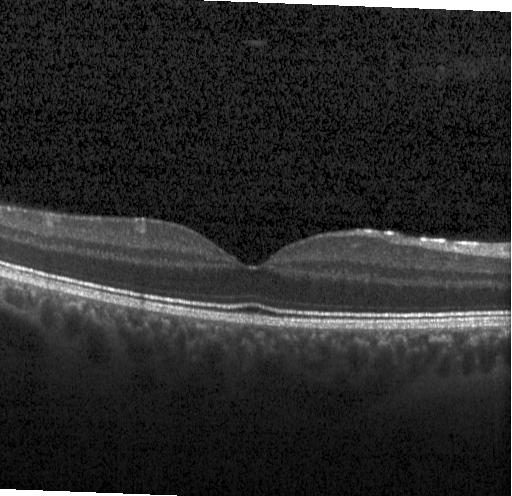

OCT B-scan; horizontal scan through the fovea. Finding: no evidence of CNV, DME, or drusen.